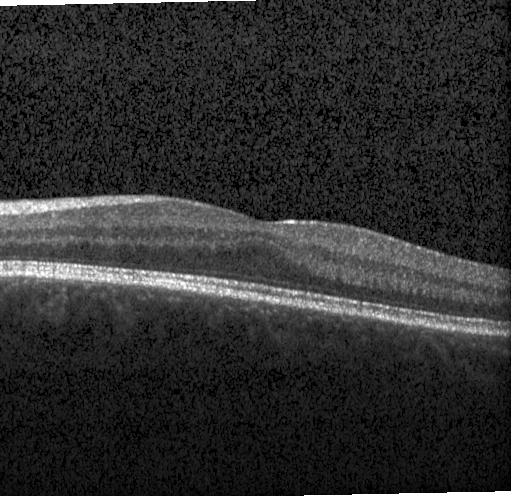

OCT B-scan; acquired on a Heidelberg Spectralis — Dx: no CNV, DME, or drusen.